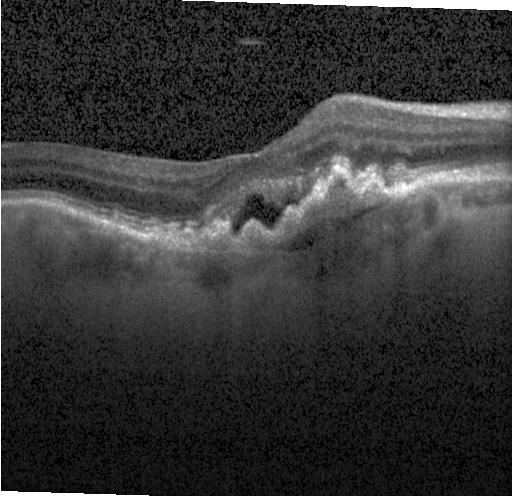

Retinal OCT B-scan · macular scan · spectral-domain OCT. Diagnosis: choroidal neovascularization.